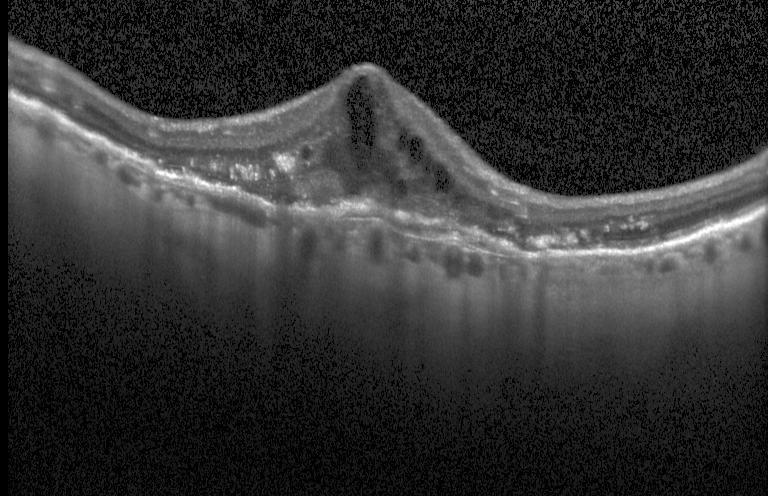

Impression: a choroidal neovascular membrane.